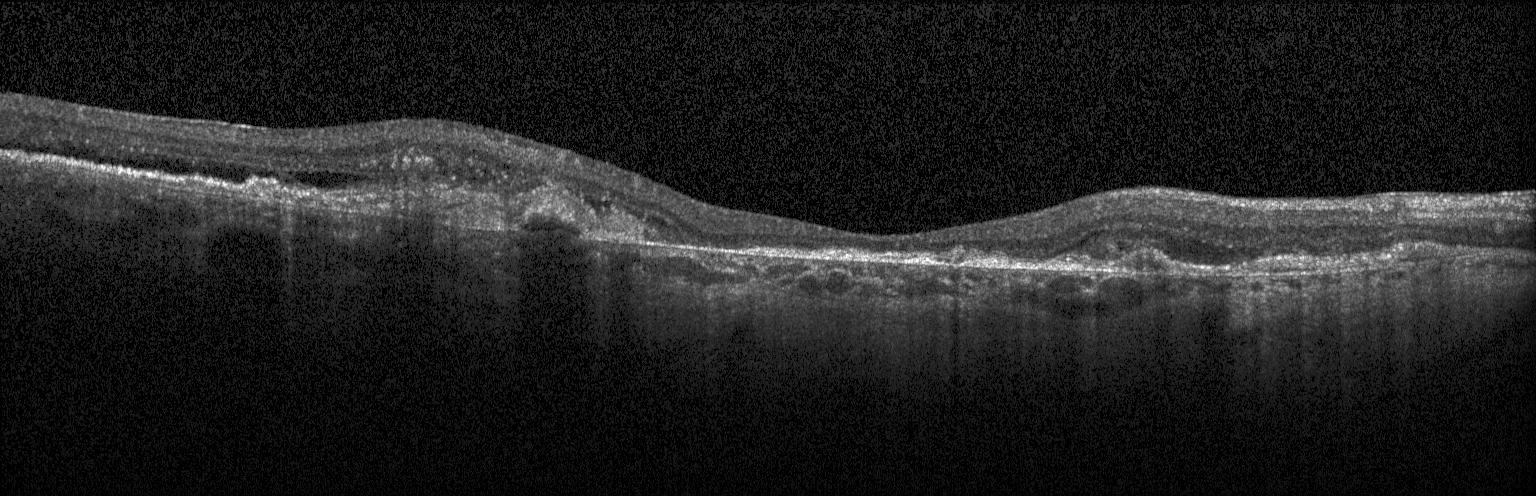
Instrument: Heidelberg Spectralis, spectral-domain optical coherence tomography, through the macula, retinal OCT B-scan — OCT finding: CNV.